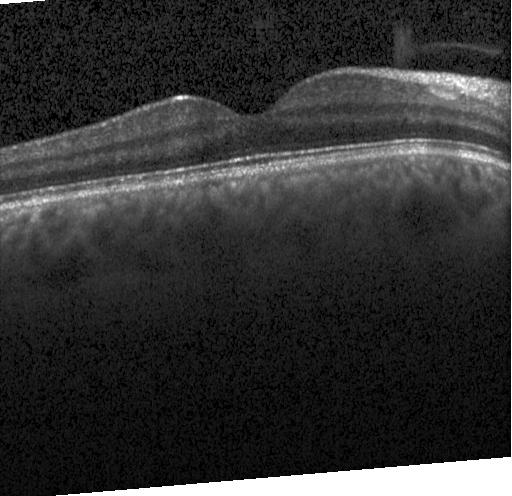

This B-scan demonstrates no choroidal neovascularization, diabetic macular edema, or drusen.